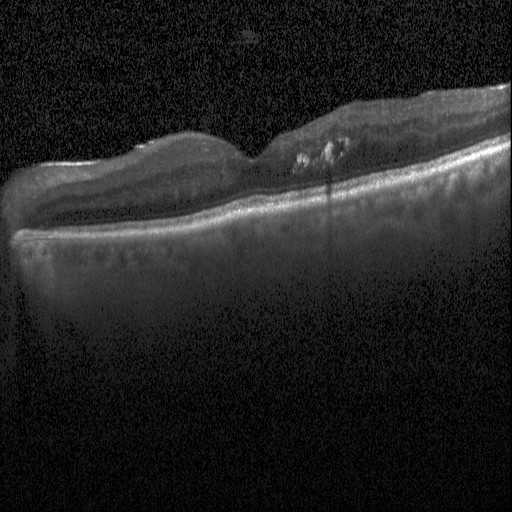
Diagnosis: diabetic macular edema (DME).